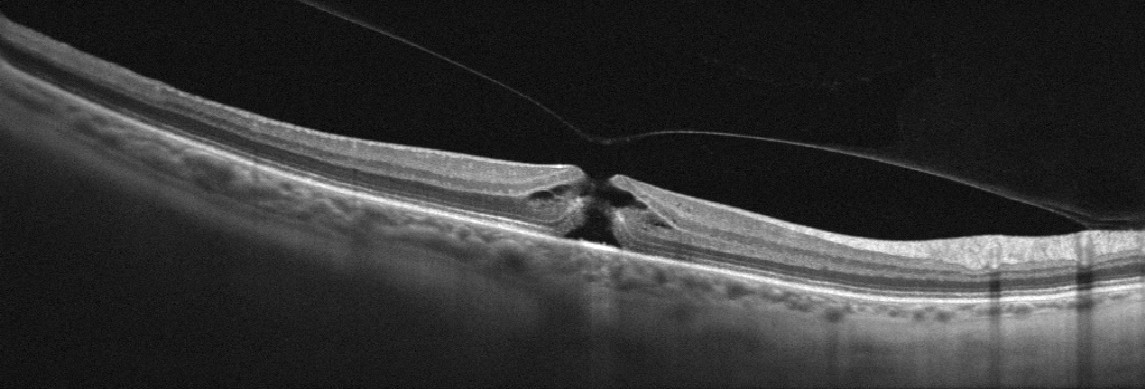

Macular scan; optical coherence tomography scan. OCT finding: vitreomacular interface disease.